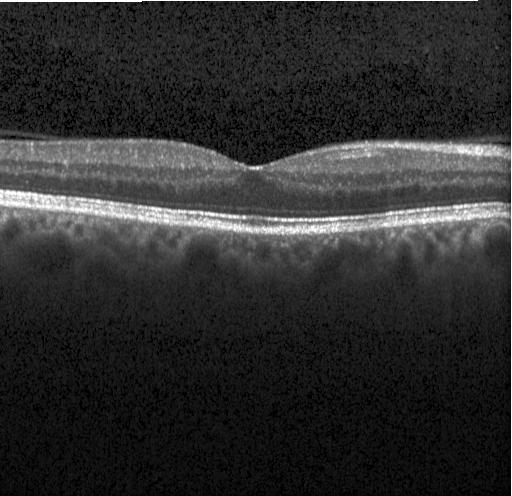

Diagnosis: no choroidal neovascularization, no diabetic macular edema, and no drusen.